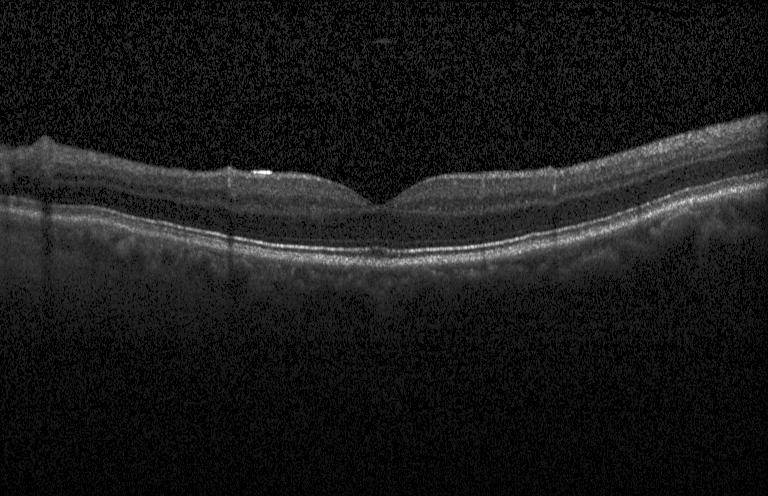
Macular OCT: no choroidal neovascularization, diabetic macular edema, or drusen.